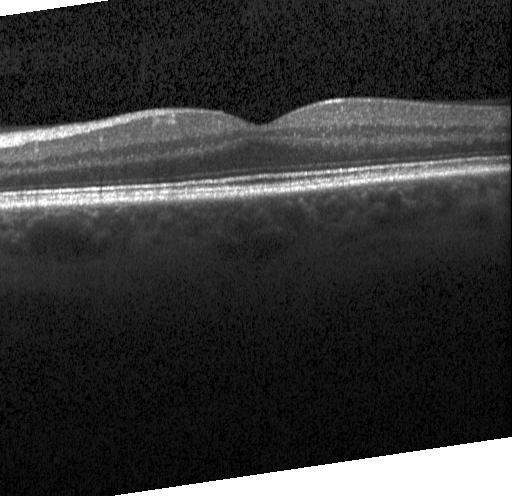
SD-OCT · through the macula · retinal OCT cross-section
No choroidal neovascularization, diabetic macular edema, or drusen.